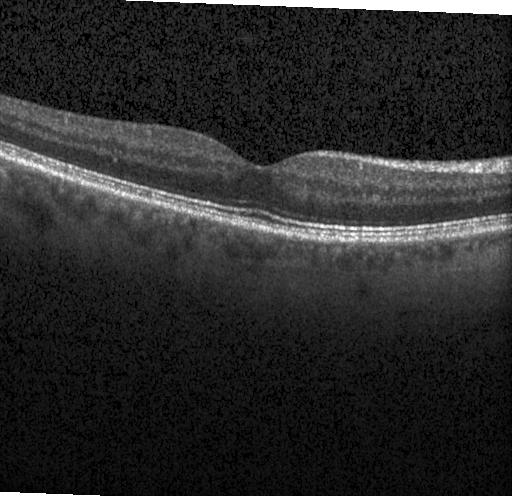
Diagnosis: no choroidal neovascularization, no diabetic macular edema, and no drusen.